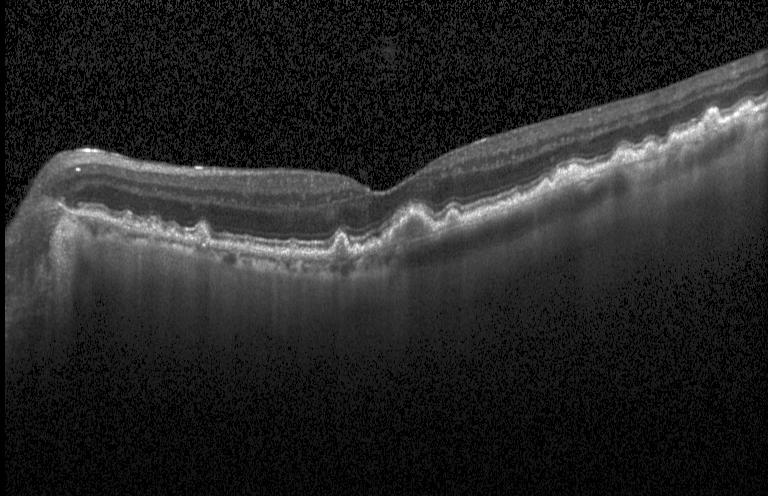
Spectral-domain optical coherence tomography. OCT B-scan. Macular scan. Finding: multiple drusen.